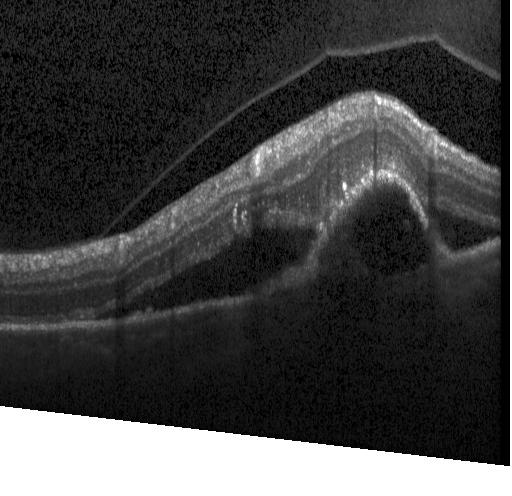
OCT B-scan, Heidelberg Spectralis, SD-OCT.
CNV.